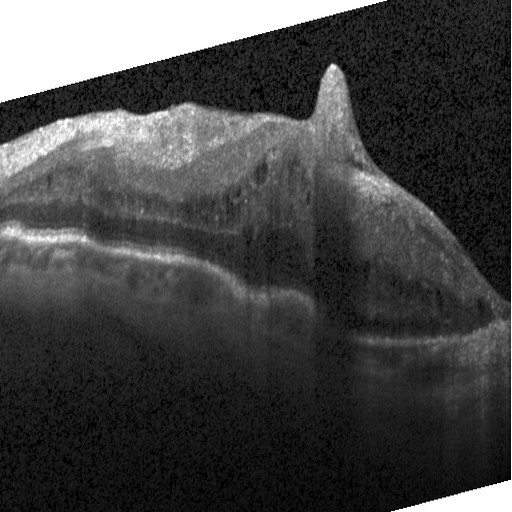

Spectral-domain optical coherence tomography, through the macula, optical coherence tomography B-scan.
Finding: diabetic macular edema (DME).